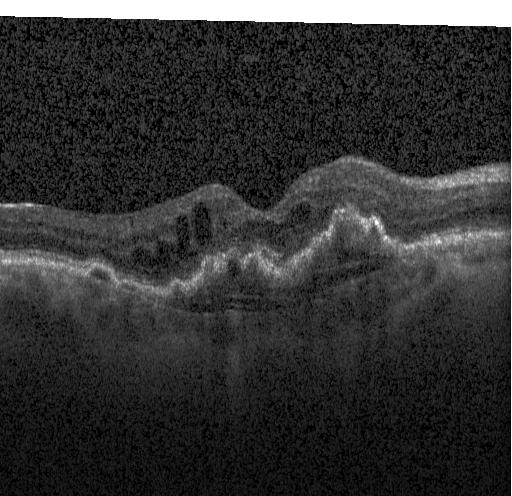

Heidelberg Spectralis · retinal OCT B-scan — This B-scan demonstrates a choroidal neovascular membrane.